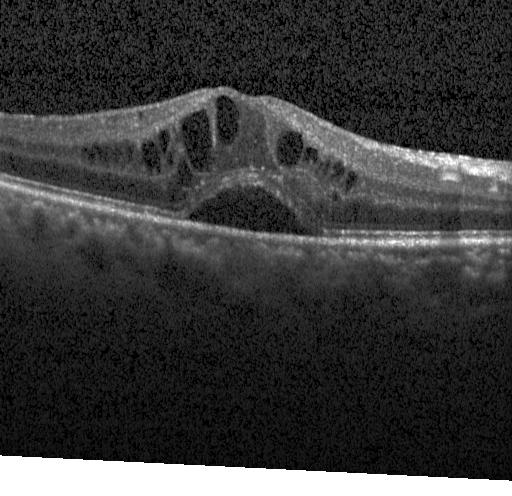

OCT finding: diabetic macular edema (DME).